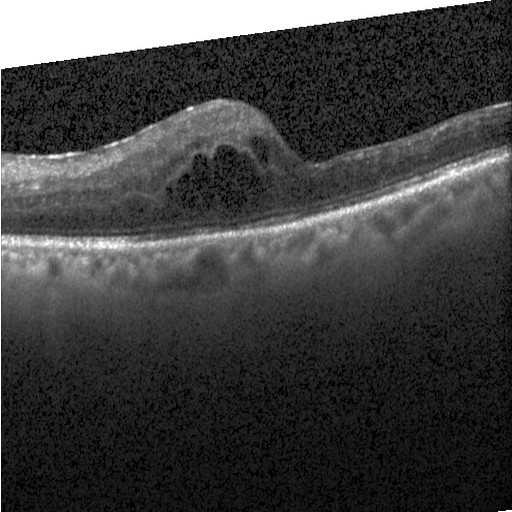 OCT B-scan
Finding: DME.